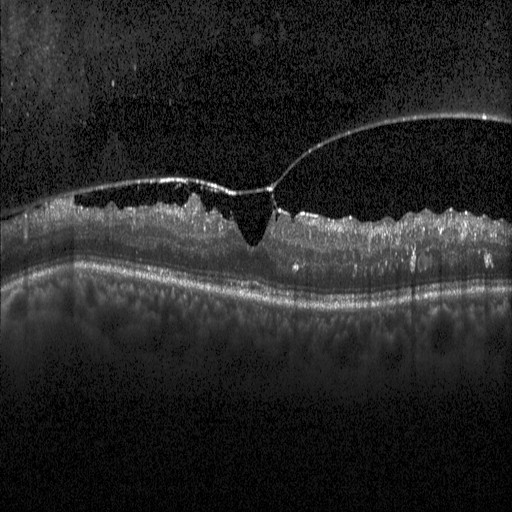 Spectral-domain OCT · OCT B-scan — Impression: diabetic macular edema (DME).